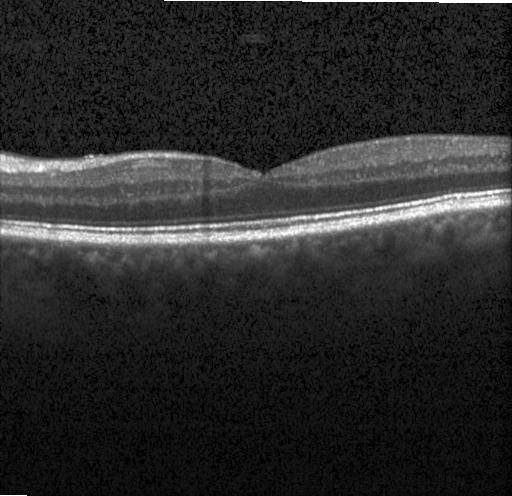

Centered on the fovea. Retinal OCT cross-section. SD-OCT. Heidelberg Spectralis.
Impression: no choroidal neovascularization, diabetic macular edema, or drusen.